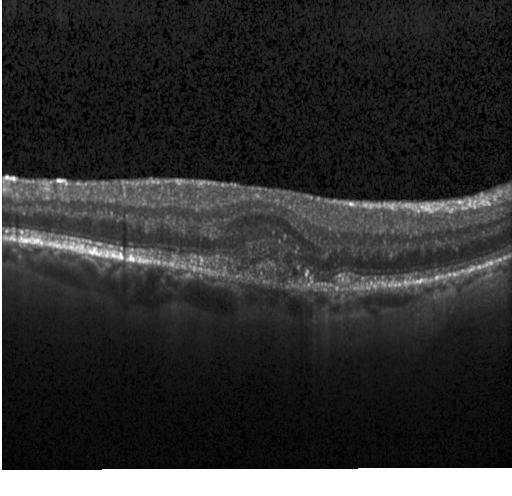

Retinal OCT cross-section showing CNV.